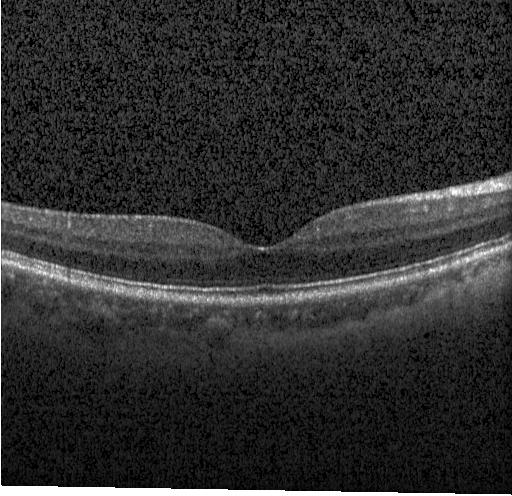
Neither choroidal neovascularization, diabetic macular edema, nor drusen.